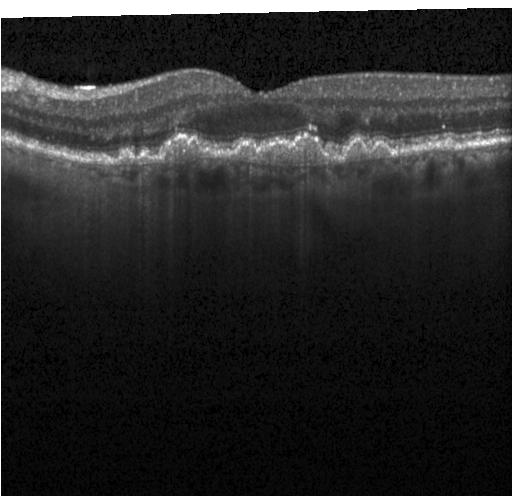

Retinal OCT cross-section showing drusen.